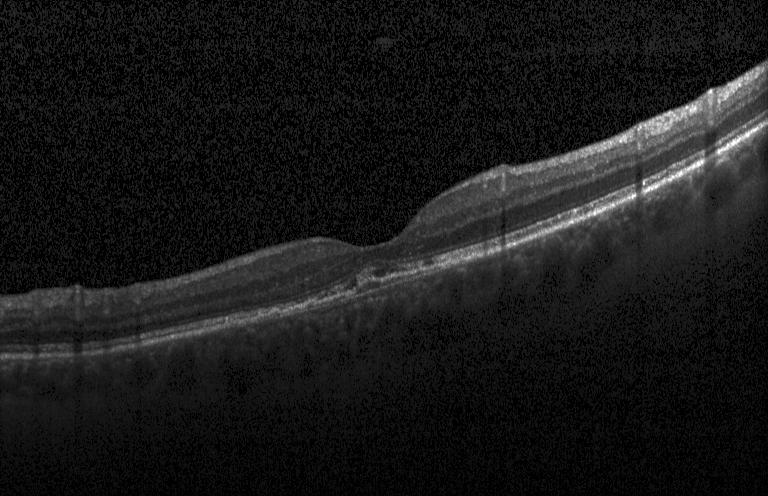

Horizontal scan through the fovea · optical coherence tomography B-scan.
Impression: choroidal neovascularization.